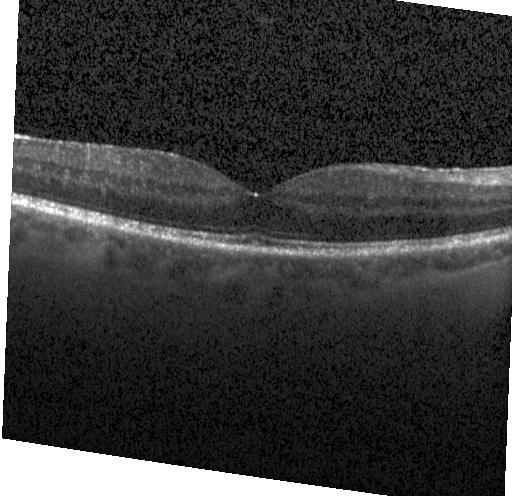

OCT line scan; Heidelberg Spectralis OCT system — Assessment: no CNV, no DME, and no drusen.